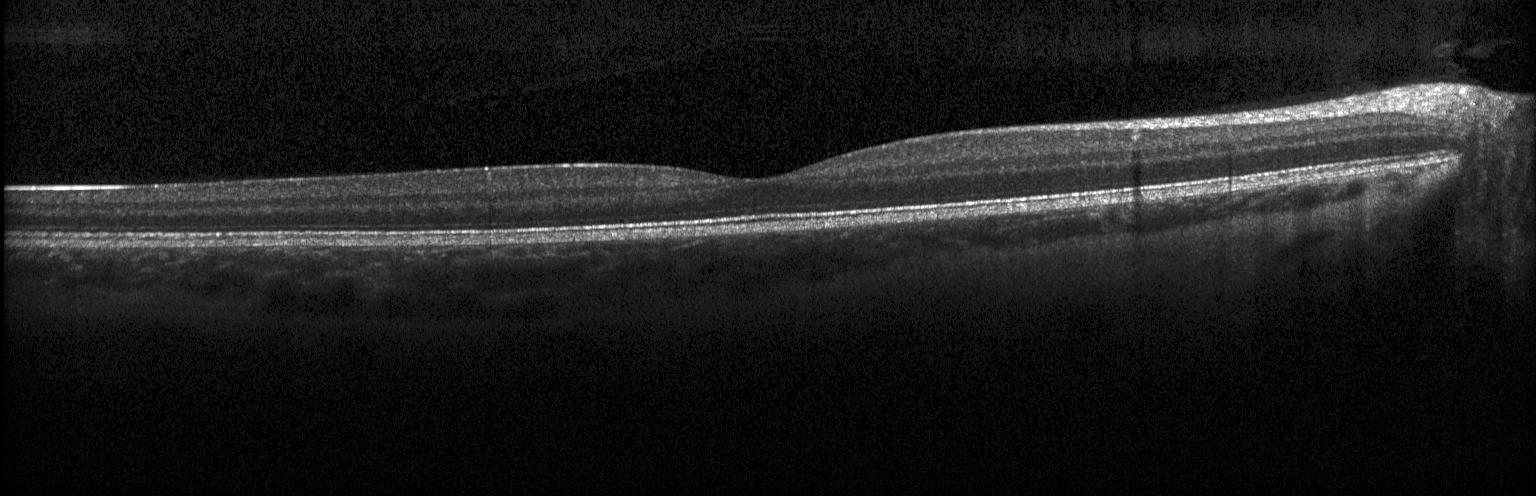

The scan shows no choroidal neovascularization, no diabetic macular edema, and no drusen.